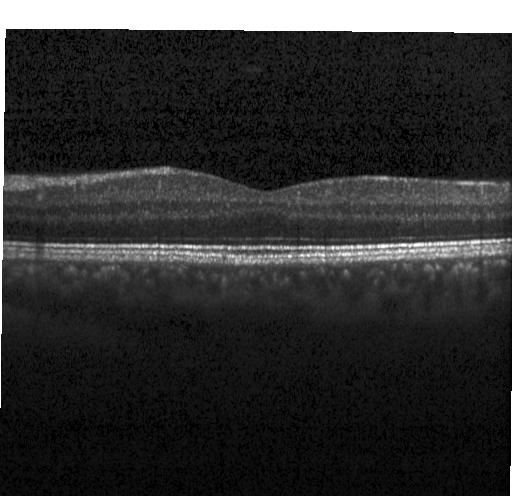
Macular OCT: no choroidal neovascularization, diabetic macular edema, or drusen.